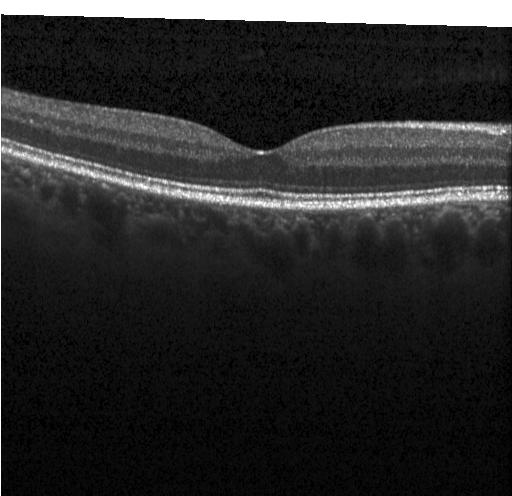

OCT B-scan
No choroidal neovascularization, diabetic macular edema, or drusen.